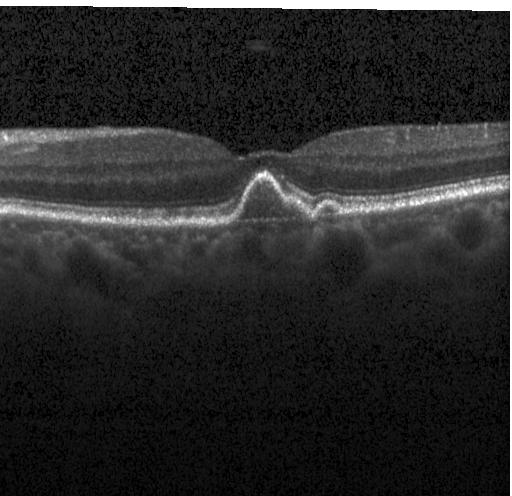

Instrument: Heidelberg Spectralis, optical coherence tomography B-scan
Finding: choroidal neovascularization (CNV).